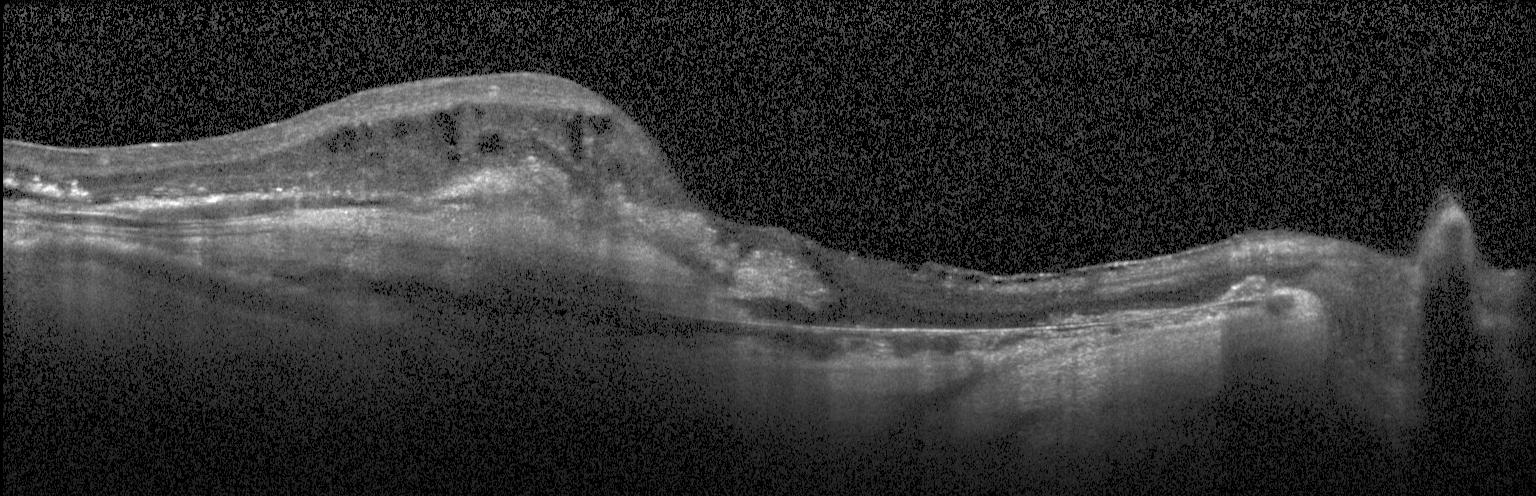
Through the macula · OCT B-scan · acquired on a Heidelberg Spectralis.
Impression: a choroidal neovascular membrane.